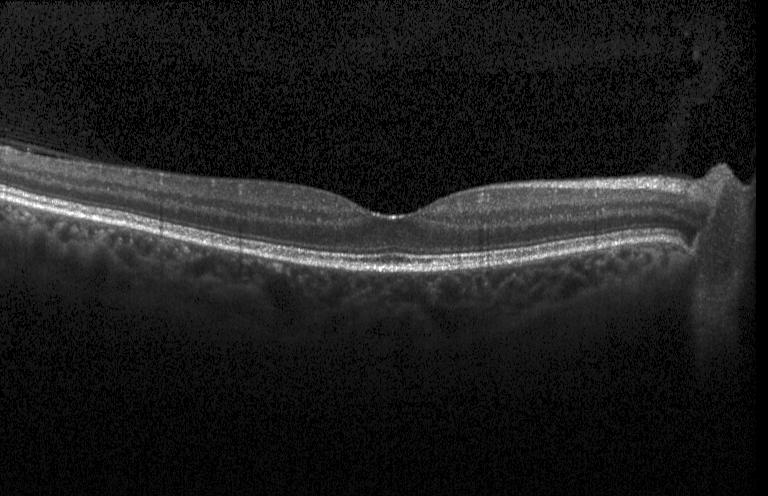 Finding: no choroidal neovascularization, no diabetic macular edema, and no drusen.